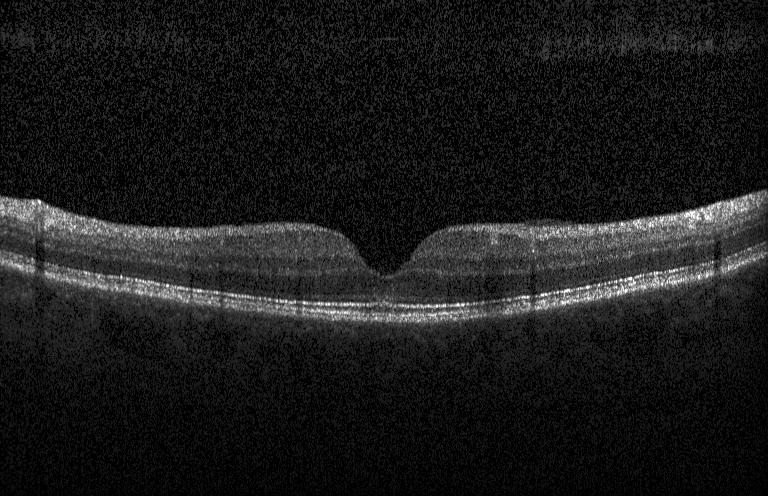
OCT finding: no choroidal neovascularization, no diabetic macular edema, and no drusen.